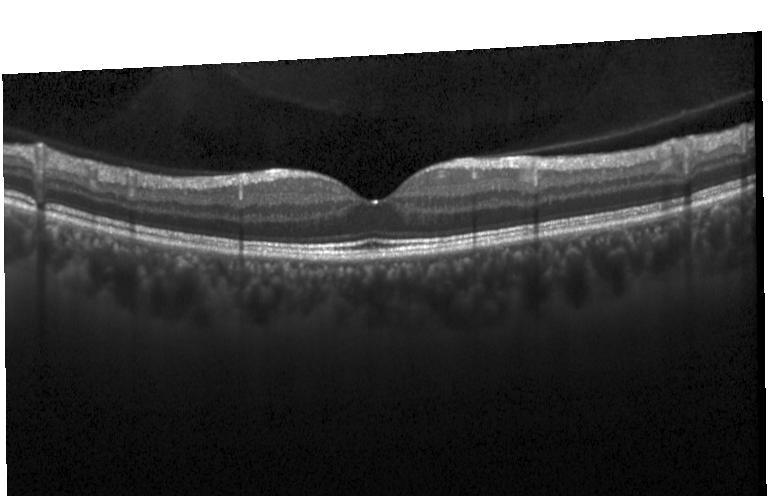

Through the macula · OCT B-scan
The scan shows no choroidal neovascularization, no diabetic macular edema, and no drusen.